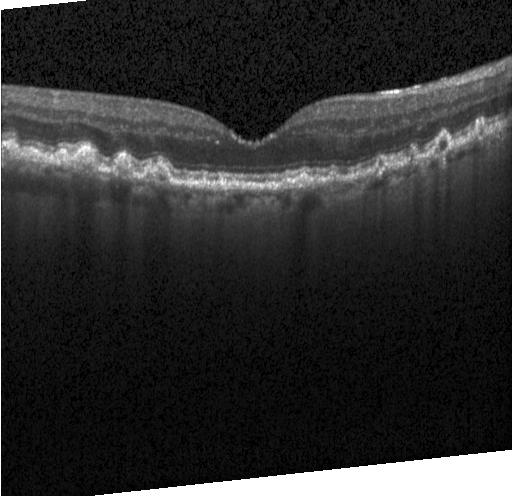
Retinal OCT cross-section
The scan shows drusen.